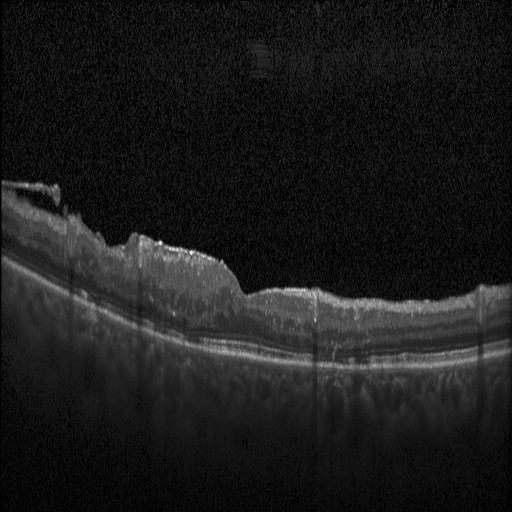 Heidelberg Spectralis OCT system; OCT B-scan. Impression: diabetic macular edema (DME).